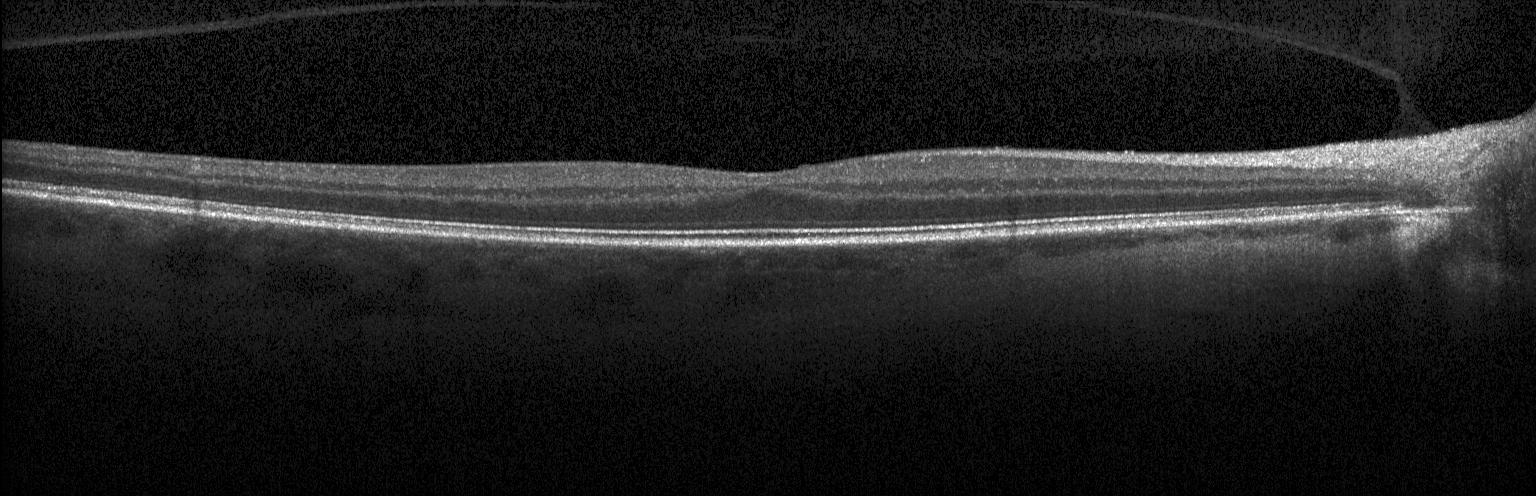 Heidelberg Spectralis OCT system. SD-OCT. Retinal OCT cross-section.
Diagnosis: no evidence of choroidal neovascularization, diabetic macular edema, or drusen.